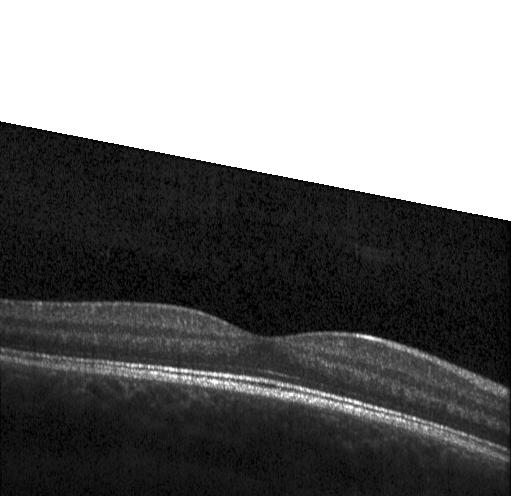

Optical coherence tomography scan. Horizontal scan through the fovea
Dx: no choroidal neovascularization, no diabetic macular edema, and no drusen.